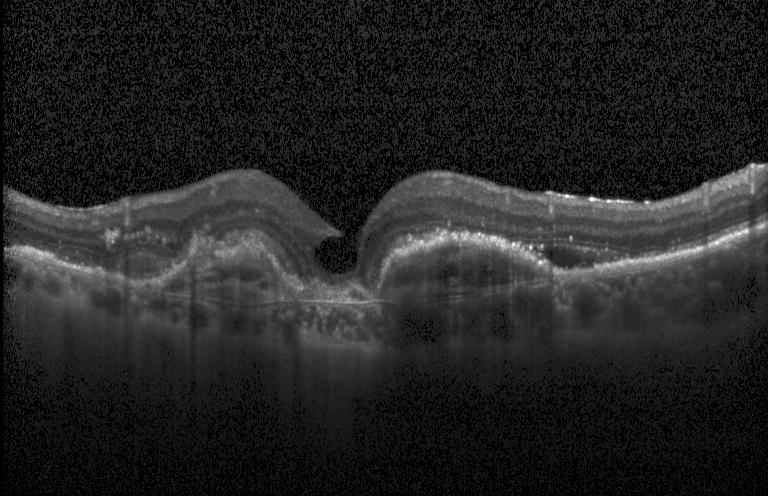

Fovea-centered. Spectral-domain optical coherence tomography. Acquired on a Heidelberg Spectralis. Optical coherence tomography scan.
Macular OCT: choroidal neovascularization.